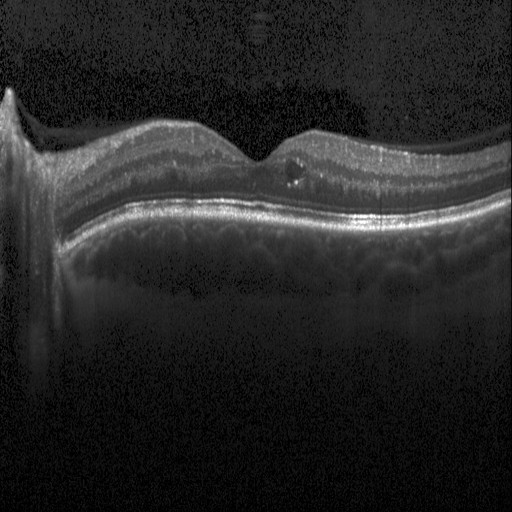

Finding: DME.